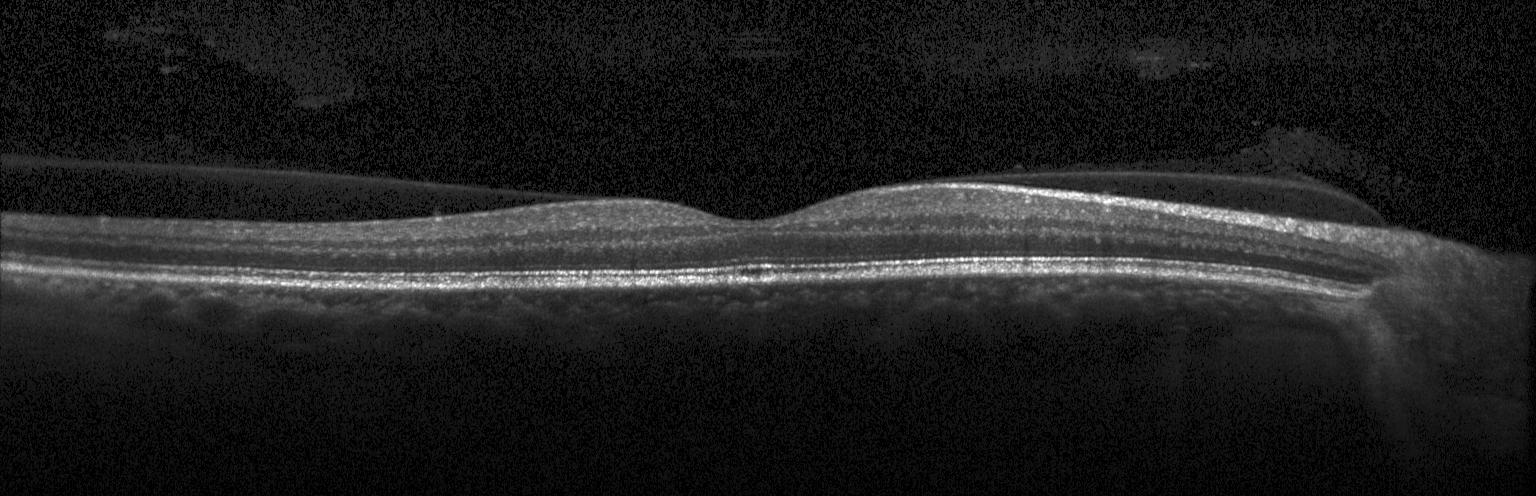

Finding: no evidence of choroidal neovascularization, diabetic macular edema, or drusen.